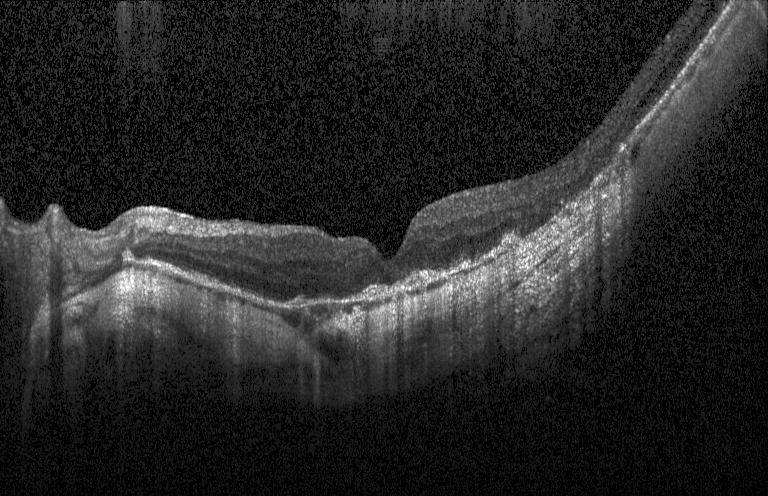

Diagnosis: CNV.